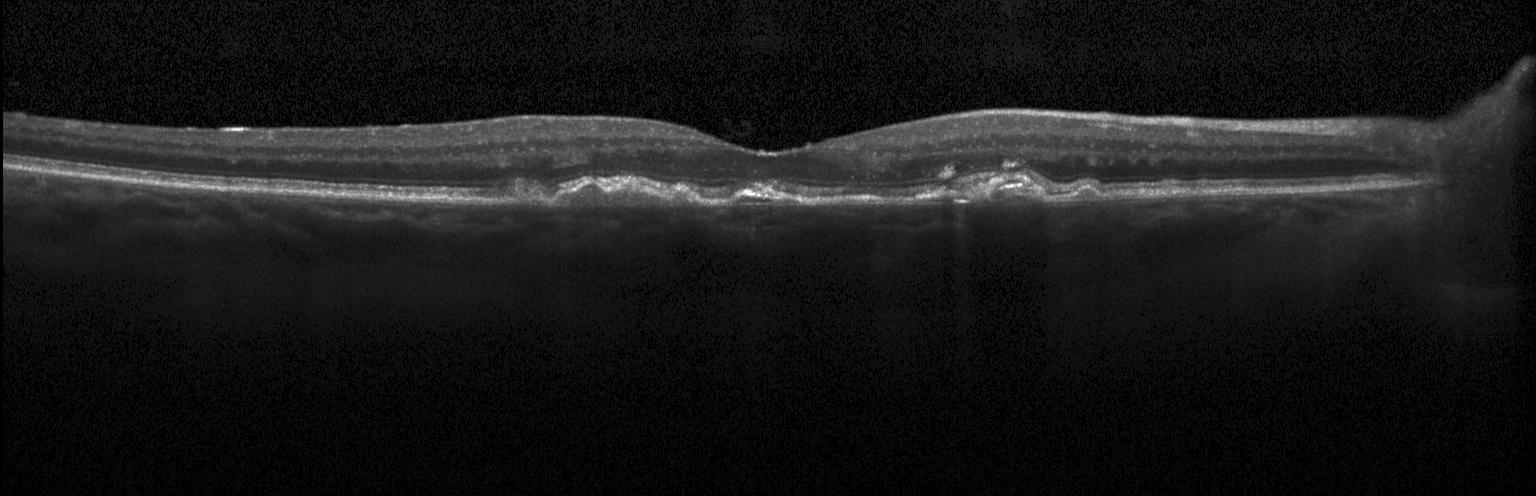
Assessment: choroidal neovascularization.